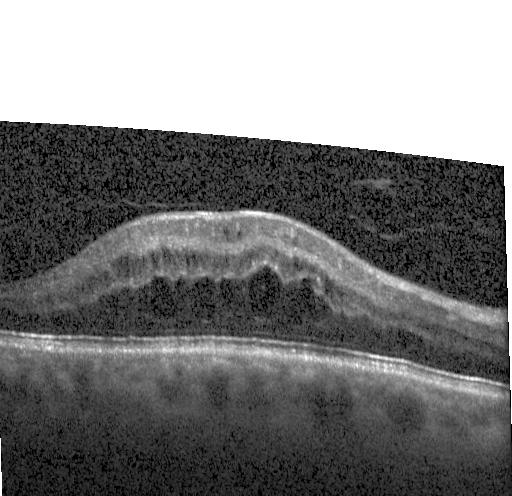
Centered on the fovea, optical coherence tomography scan — Assessment: DME.